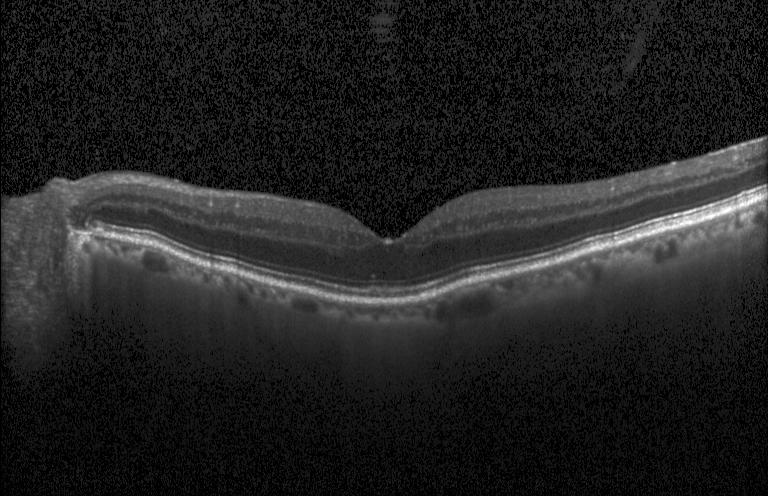

Impression: no choroidal neovascularization, diabetic macular edema, or drusen.